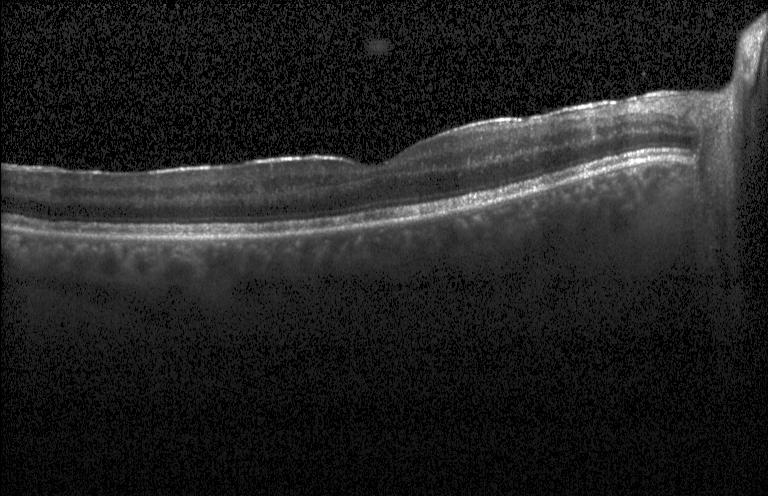

OCT line scan · centered on the fovea · acquired on a Heidelberg Spectralis.
Impression: no evidence of choroidal neovascularization, diabetic macular edema, or drusen.